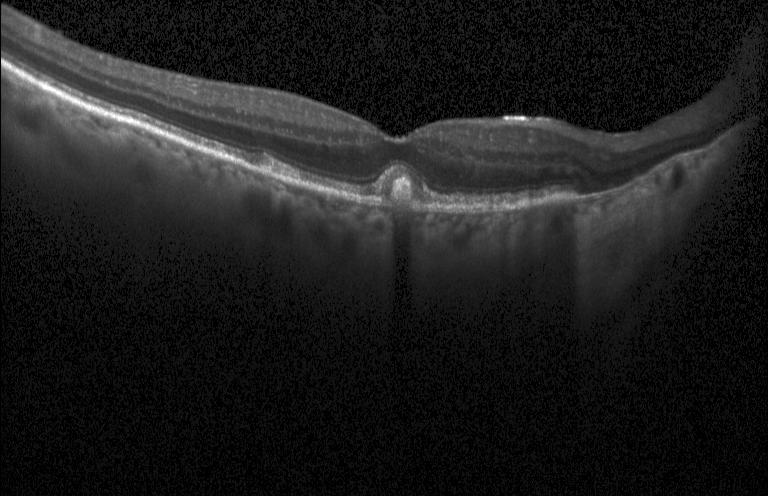

Instrument: Heidelberg Spectralis. Retinal OCT B-scan. Fovea-centered. Spectral-domain OCT
Impression: a choroidal neovascular membrane.